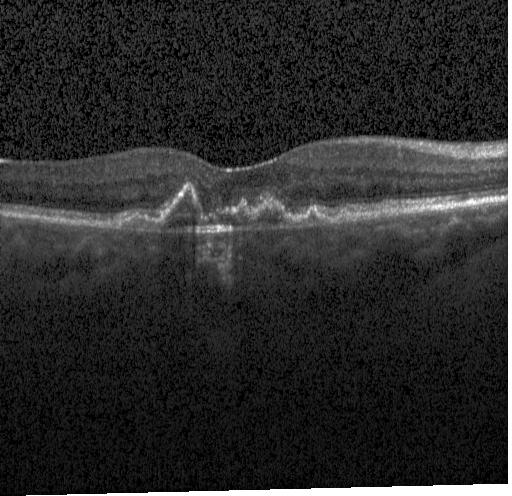

Impression: choroidal neovascularization.